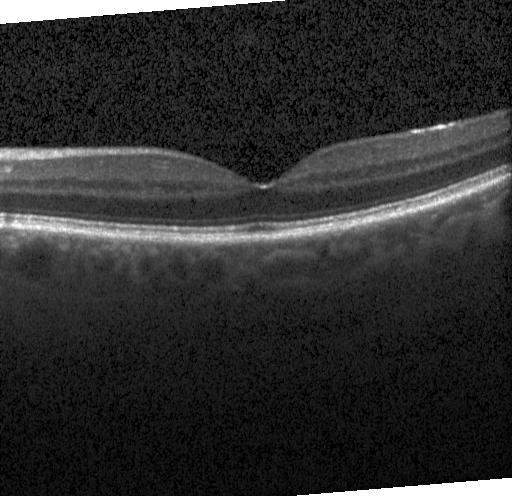 SD-OCT; Heidelberg Spectralis; through the macula; optical coherence tomography scan.
Finding: no evidence of CNV, DME, or drusen.